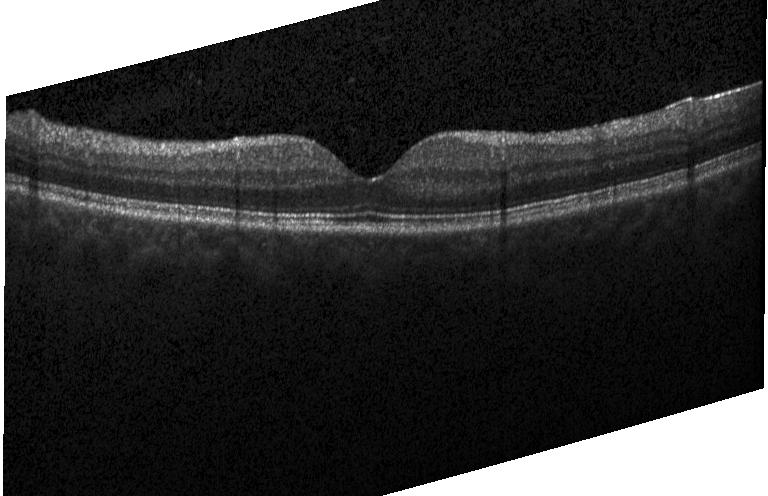
OCT B-scan, Heidelberg Spectralis OCT system, spectral-domain OCT. Impression: no CNV, DME, or drusen.